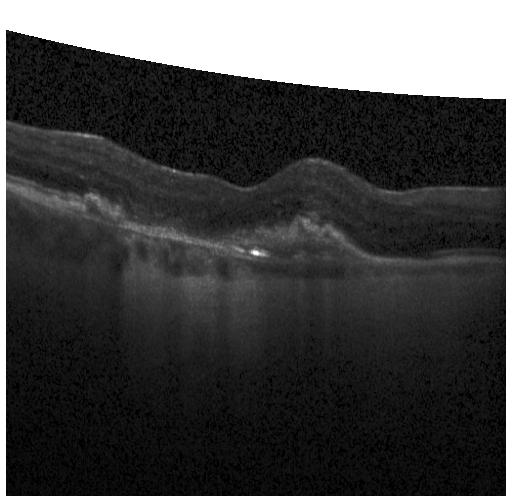 Macular scan. Retinal OCT cross-section. Heidelberg Spectralis — This B-scan demonstrates a choroidal neovascular membrane.